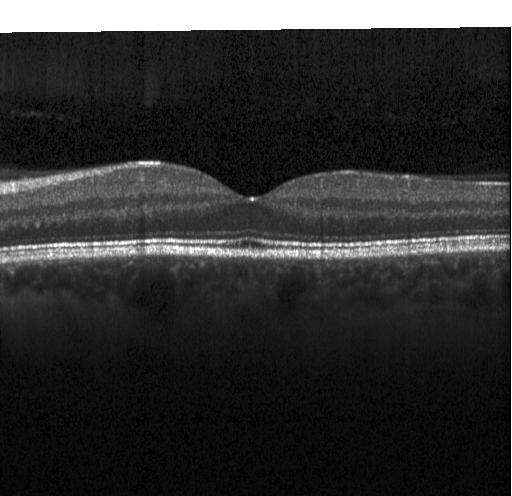 Dx: no evidence of CNV, DME, or drusen.